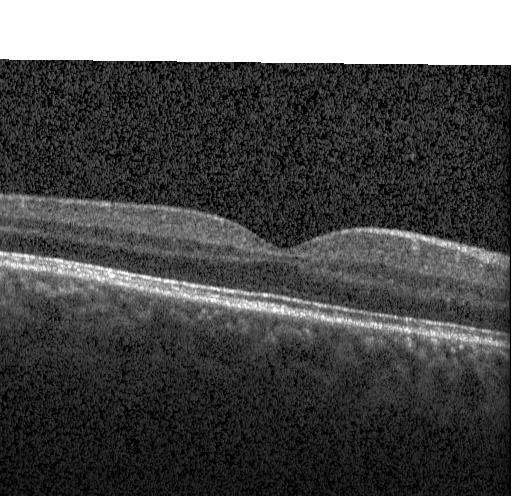
Diagnosis: no CNV, no DME, and no drusen.